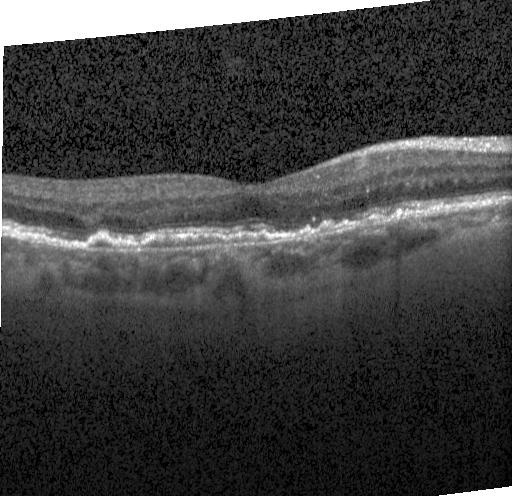
OCT B-scan showing a choroidal neovascular membrane.